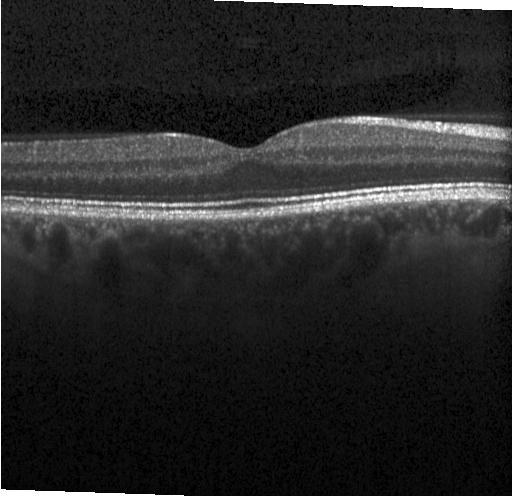
Diagnosis: no CNV, no DME, and no drusen.